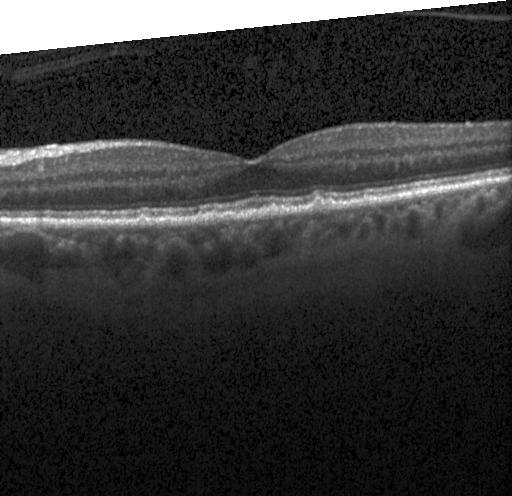
Spectral-domain optical coherence tomography; retinal OCT B-scan; through the macula.
Finding: sub-RPE drusenoid deposits.